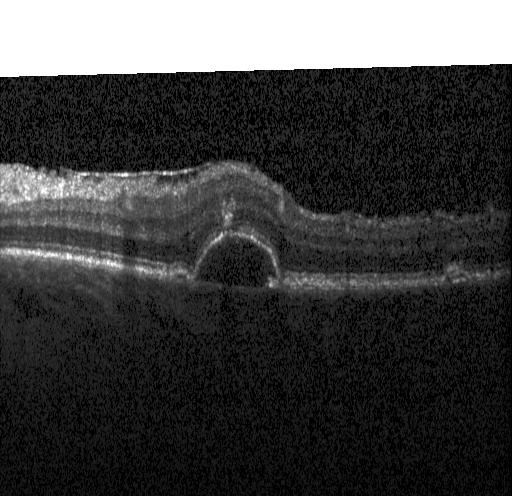

Retinal OCT cross-section, centered on the fovea
Diagnosis: CNV.